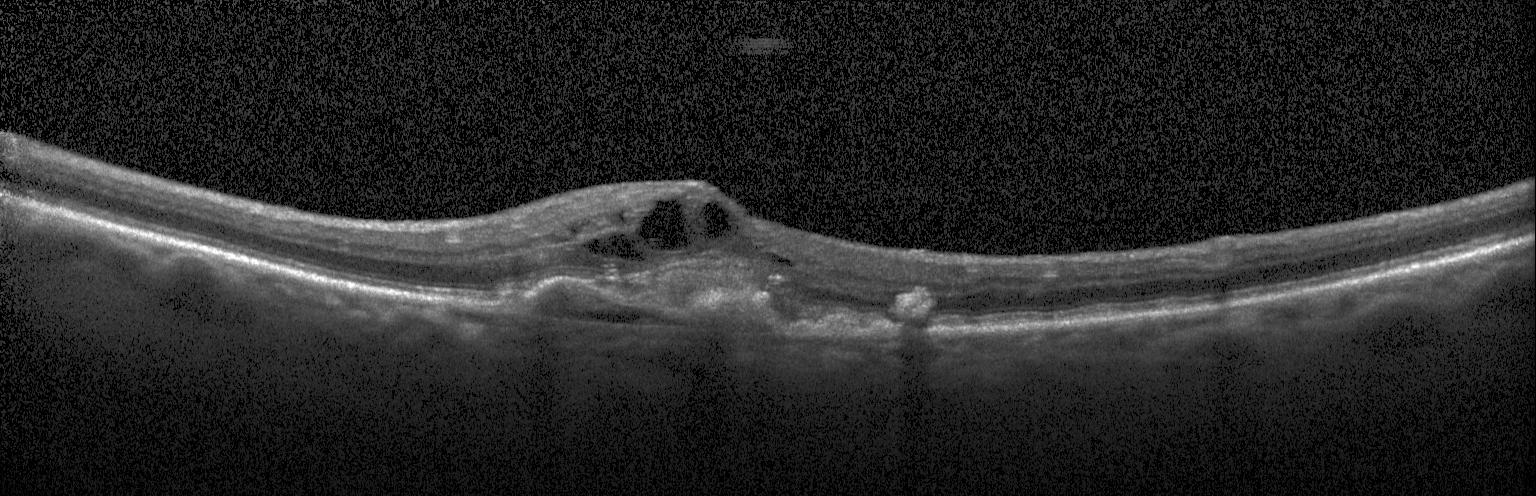 Impression: CNV.